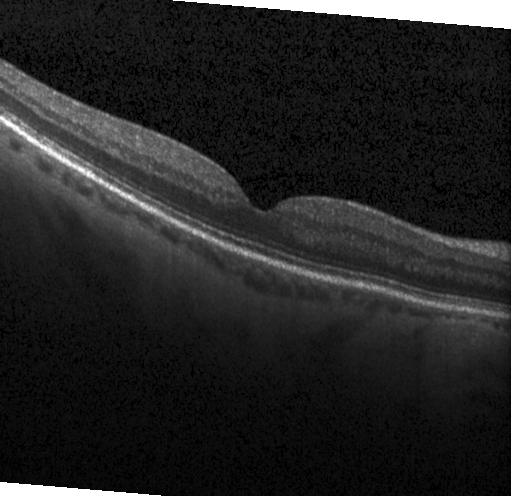
Retinal OCT cross-section.
Macular OCT: no evidence of choroidal neovascularization, diabetic macular edema, or drusen.